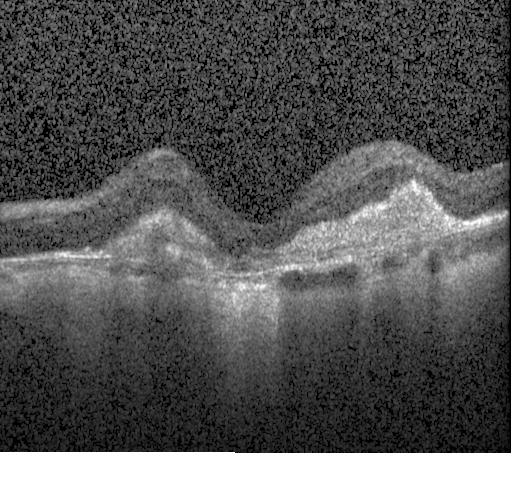
Retinal OCT cross-section. Centered on the fovea. Spectral-domain optical coherence tomography. Acquired on a Heidelberg Spectralis — This B-scan demonstrates a choroidal neovascular membrane.